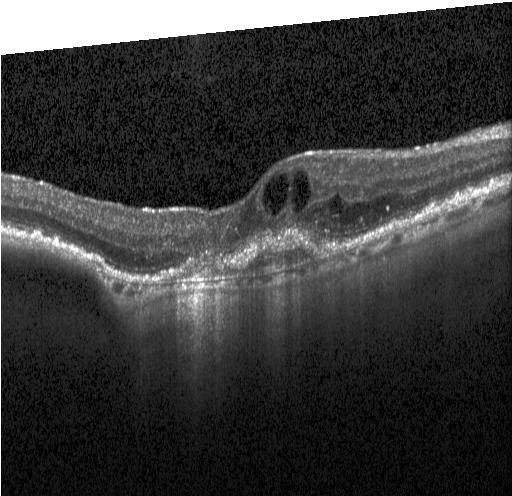
Acquired on a Heidelberg Spectralis · spectral-domain optical coherence tomography · fovea-centered · retinal OCT B-scan. OCT finding: choroidal neovascularization (CNV).